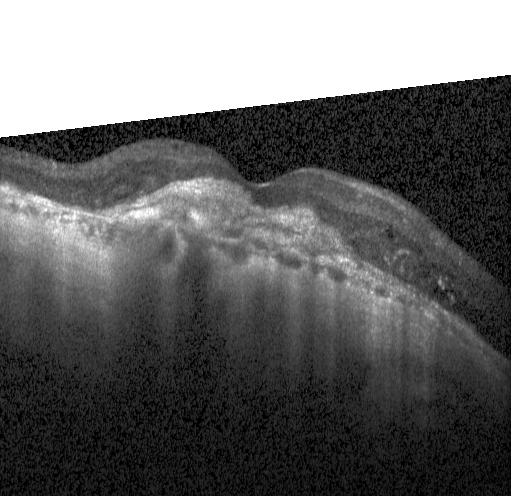

Diagnosis: a choroidal neovascular membrane.